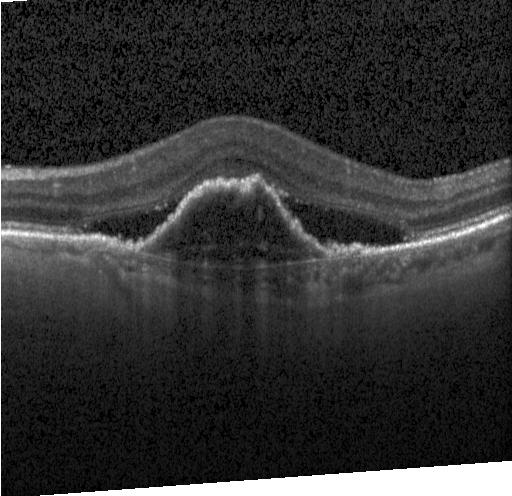 Optical coherence tomography B-scan.
Finding: a choroidal neovascular membrane.